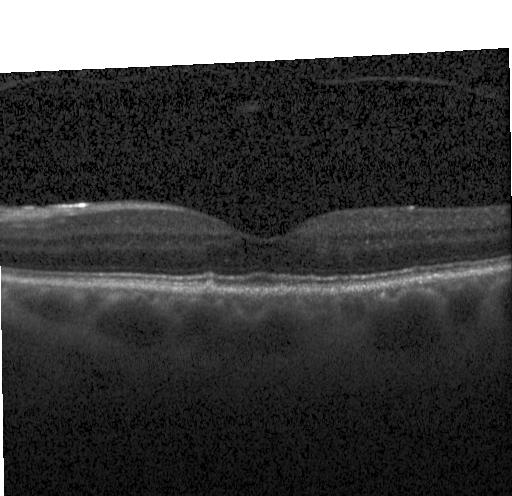
Retinal OCT B-scan · spectral-domain OCT · Heidelberg Spectralis OCT system.
Macular OCT: sub-RPE drusenoid deposits.